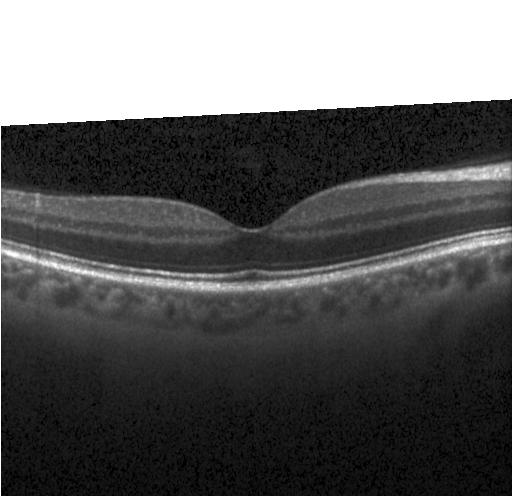
Dx: no evidence of choroidal neovascularization, diabetic macular edema, or drusen.